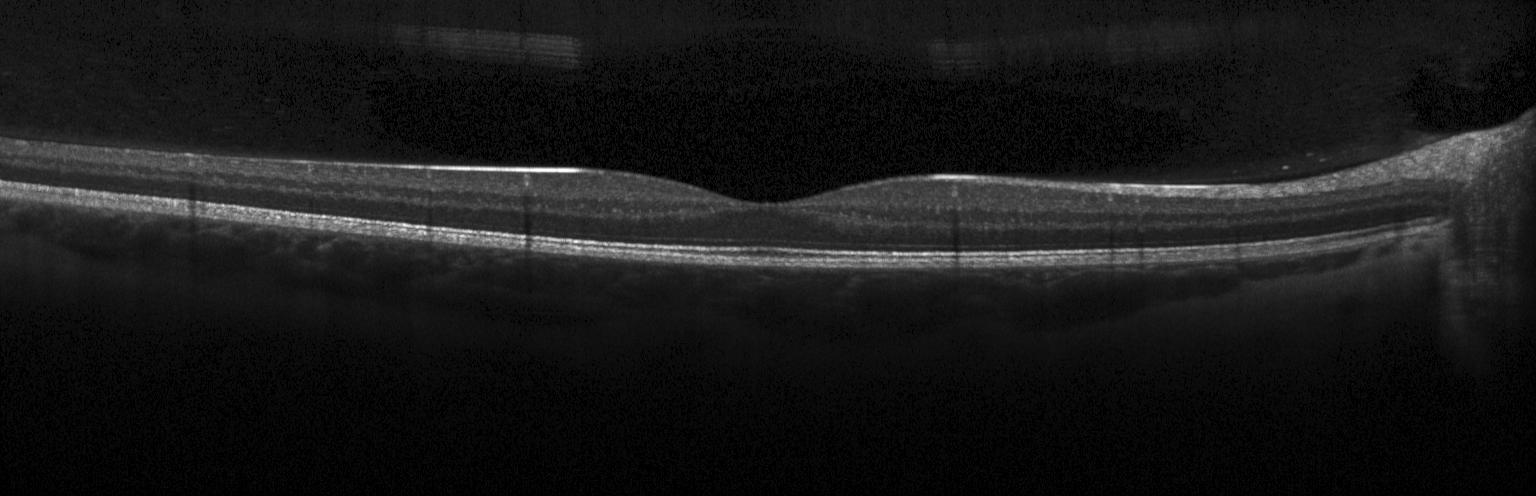
Spectral-domain optical coherence tomography · OCT line scan · macular scan · instrument: Heidelberg Spectralis.
This B-scan demonstrates no CNV, DME, or drusen.